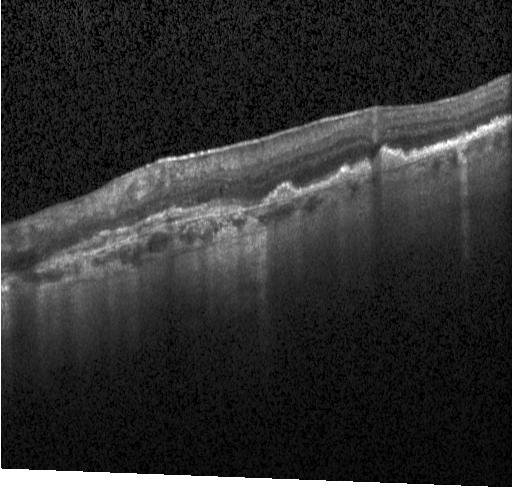
Retinal OCT cross-section. Impression: a choroidal neovascular membrane.